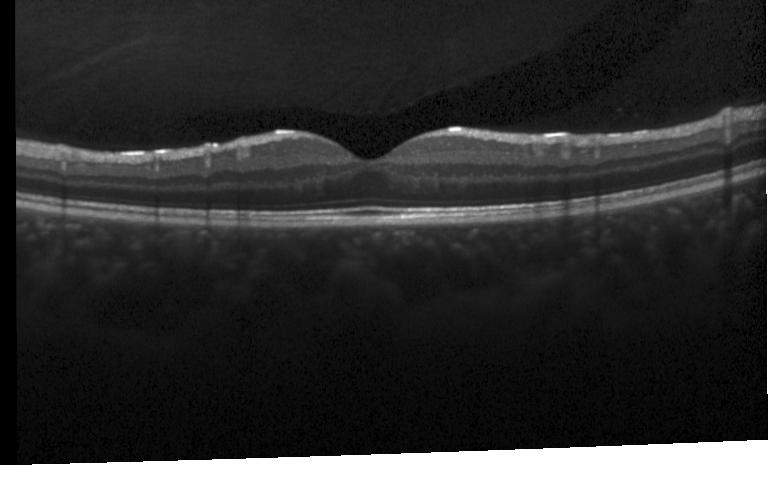
This B-scan demonstrates no evidence of choroidal neovascularization, diabetic macular edema, or drusen.